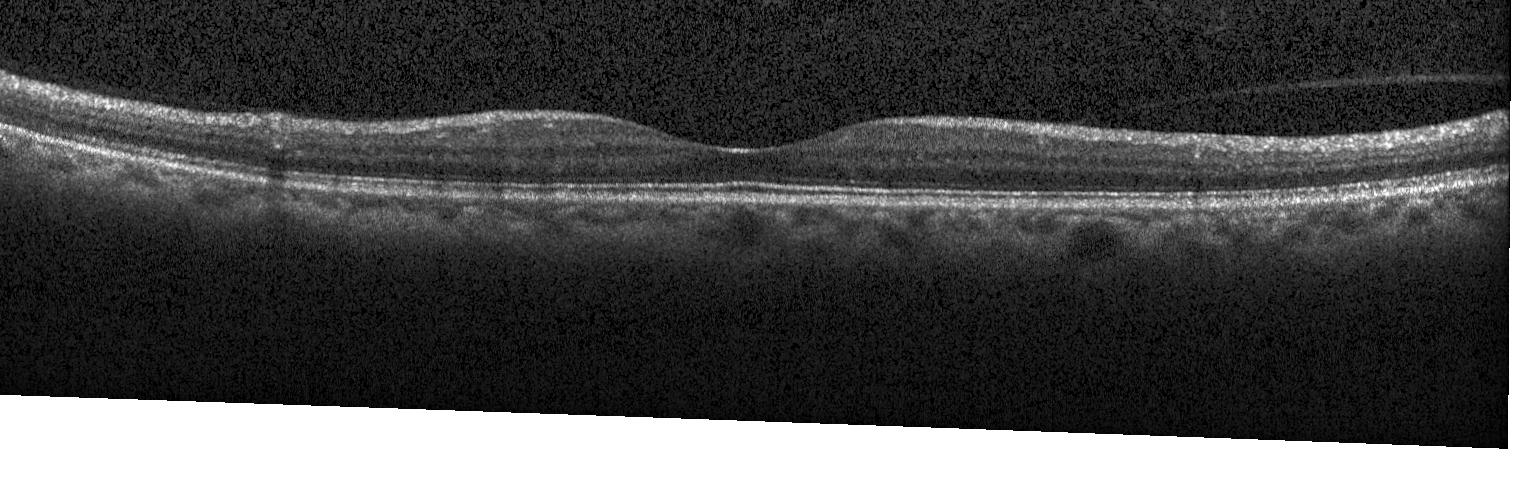 Optical coherence tomography scan, acquired on a Heidelberg Spectralis, spectral-domain OCT — Impression: neither choroidal neovascularization, diabetic macular edema, nor drusen.